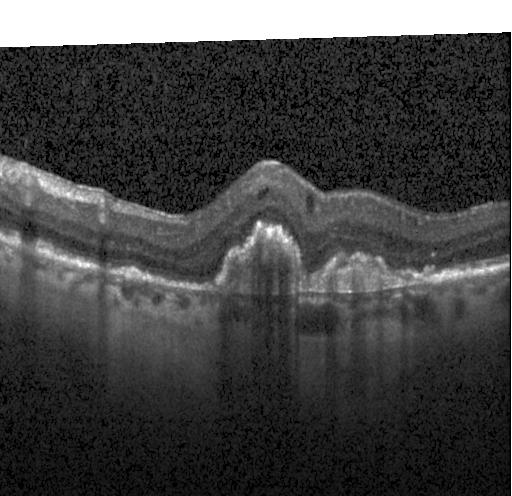

SD-OCT. Retinal OCT cross-section. Horizontal scan through the fovea. Heidelberg Spectralis
Assessment: choroidal neovascularization.